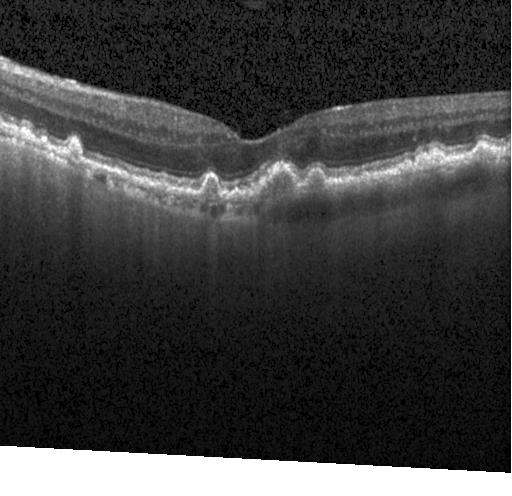 Finding: multiple drusen.